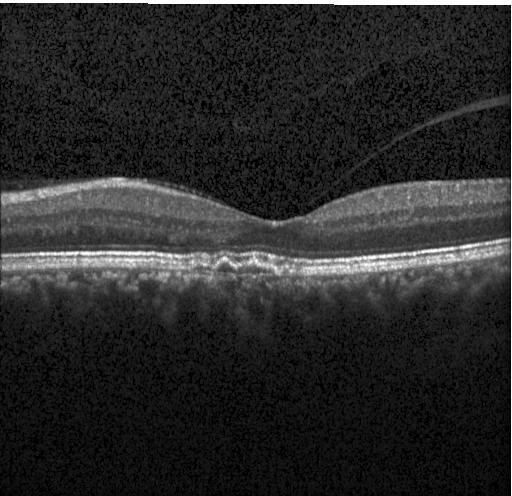

Macular OCT: multiple drusen.